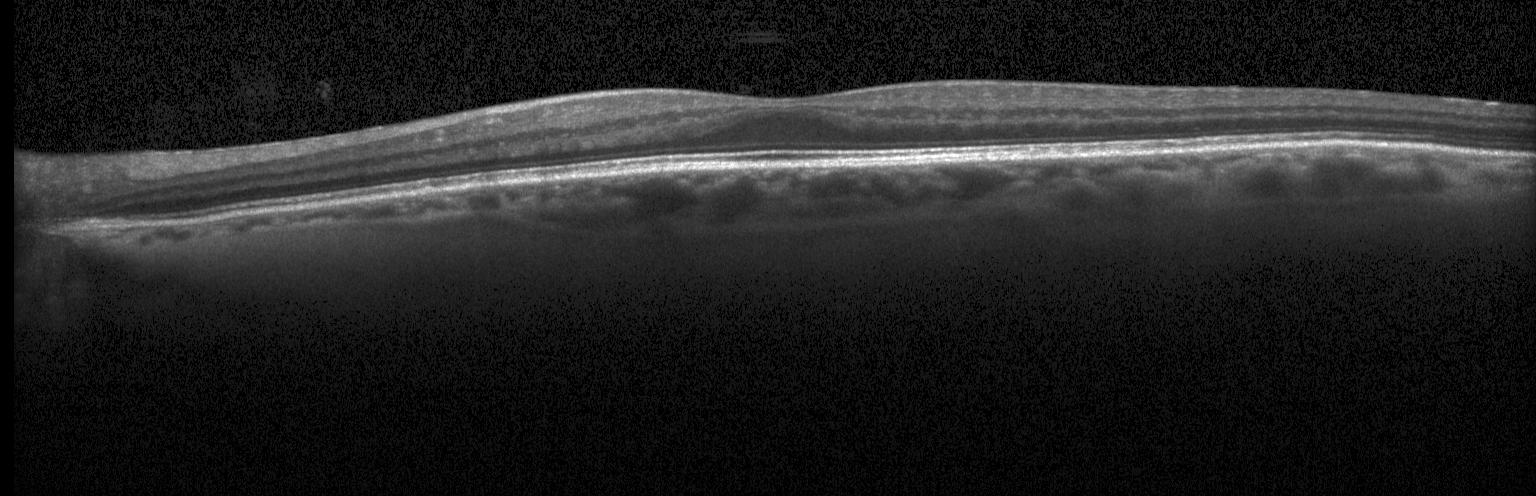

Through the macula. OCT line scan. Spectral-domain OCT — Dx: no evidence of CNV, DME, or drusen.